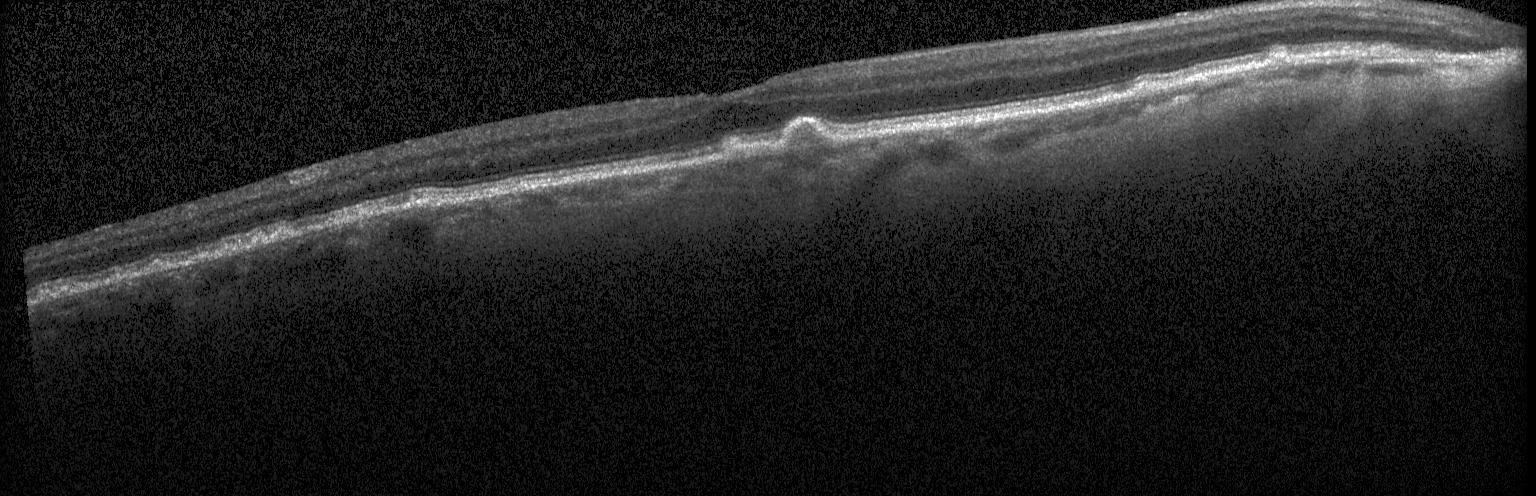 Instrument: Heidelberg Spectralis. OCT B-scan.
Impression: multiple drusen.